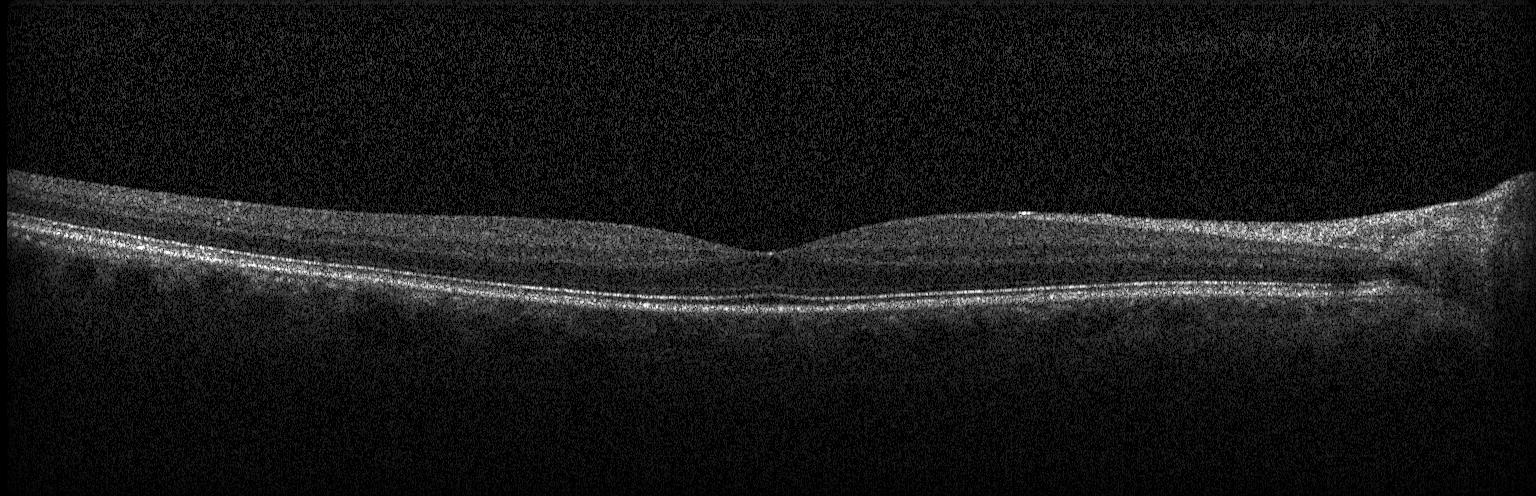 Optical coherence tomography scan — Dx: neither choroidal neovascularization, diabetic macular edema, nor drusen.